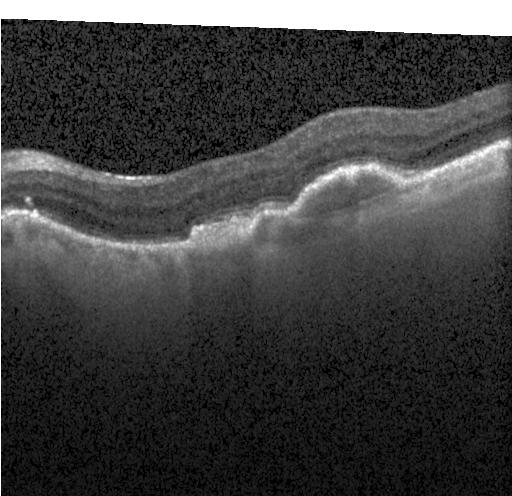

OCT line scan · SD-OCT · Heidelberg Spectralis · horizontal scan through the fovea
Impression: choroidal neovascularization.